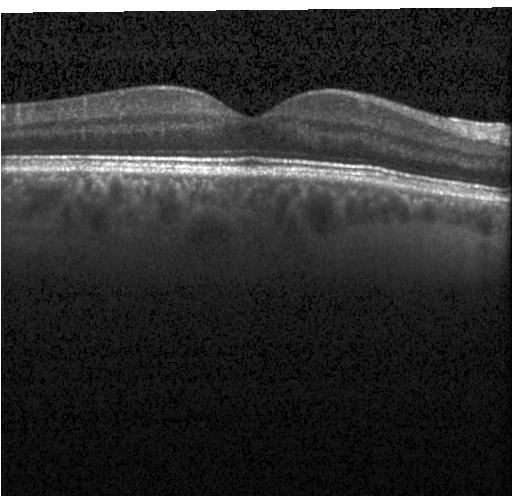 This B-scan demonstrates neither CNV, DME, nor drusen.